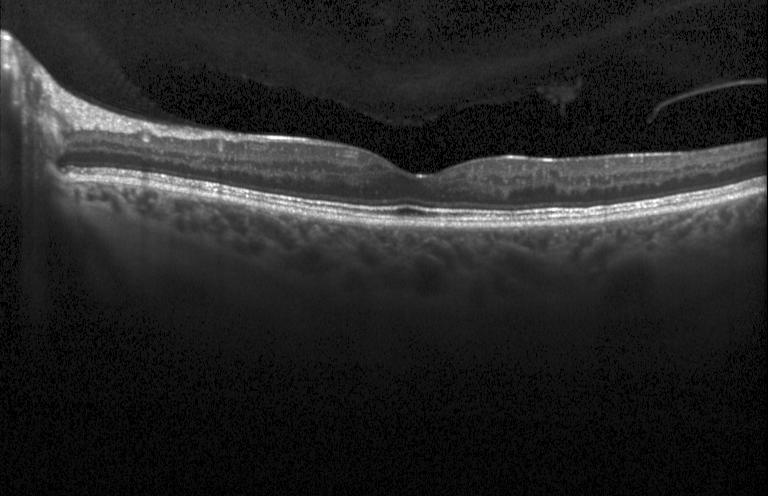 Assessment: neither choroidal neovascularization, diabetic macular edema, nor drusen.